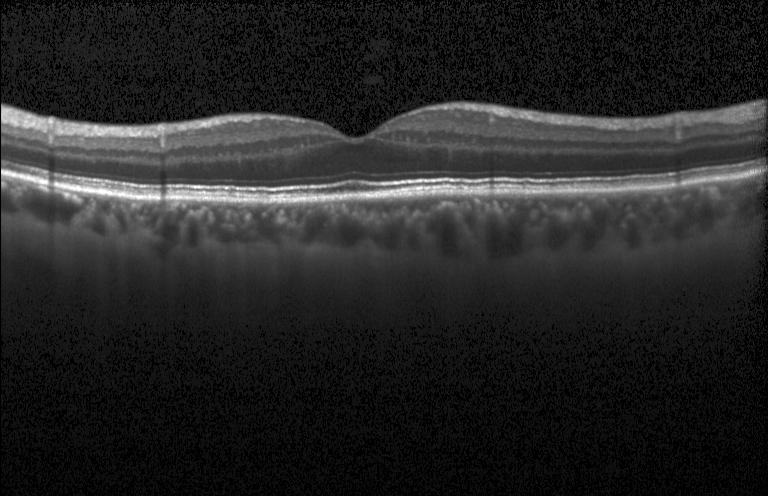

Retinal OCT cross-section, through the macula — Assessment: no choroidal neovascularization, diabetic macular edema, or drusen.